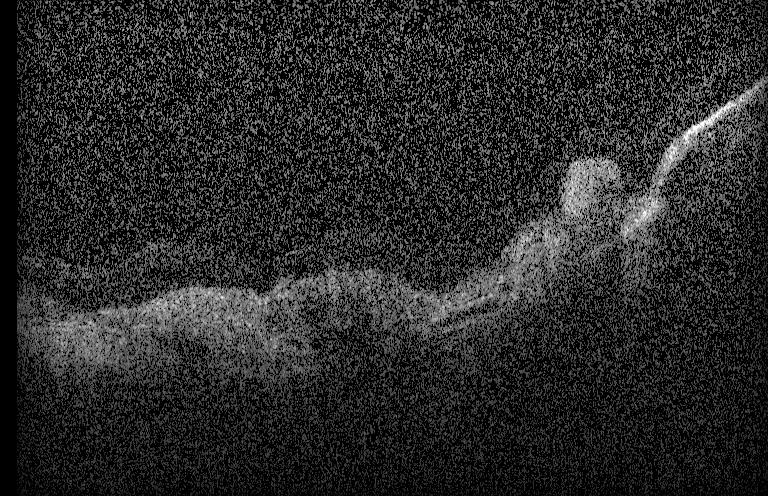
Retinal OCT B-scan, through the macula.
Finding: choroidal neovascularization (CNV).